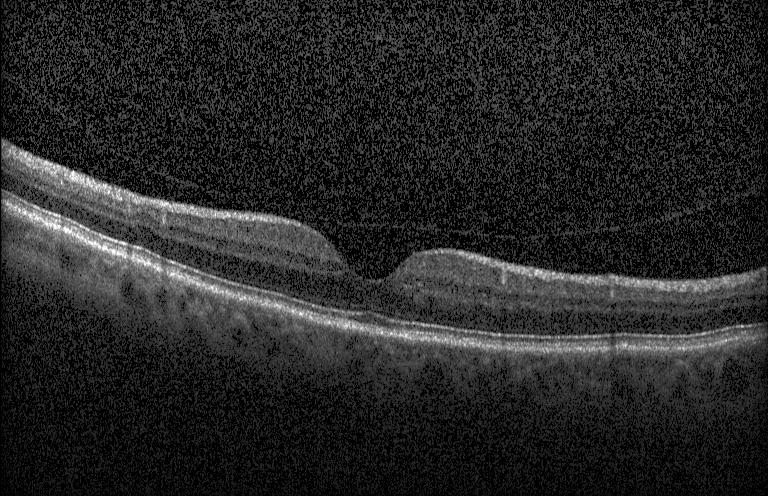

OCT line scan — Assessment: neither choroidal neovascularization, diabetic macular edema, nor drusen.